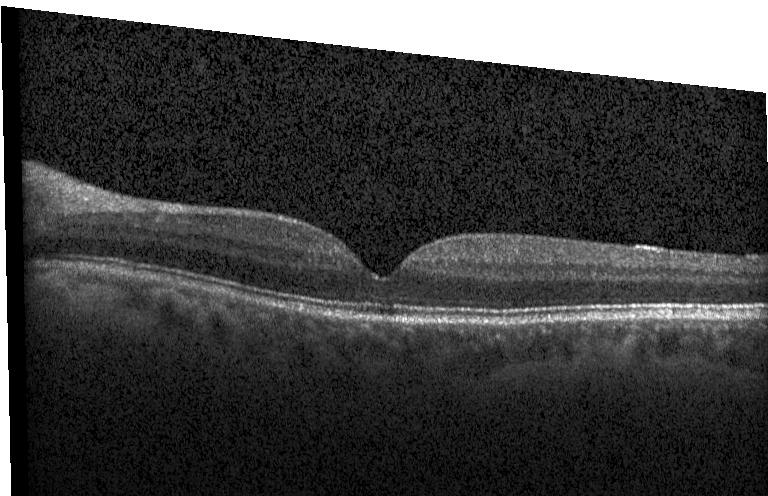 Optical coherence tomography scan; SD-OCT; macular scan. Diagnosis: no choroidal neovascularization, diabetic macular edema, or drusen.